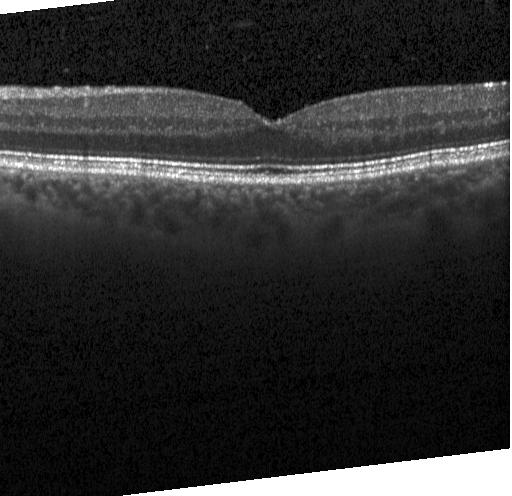

Finding: no CNV, no DME, and no drusen.